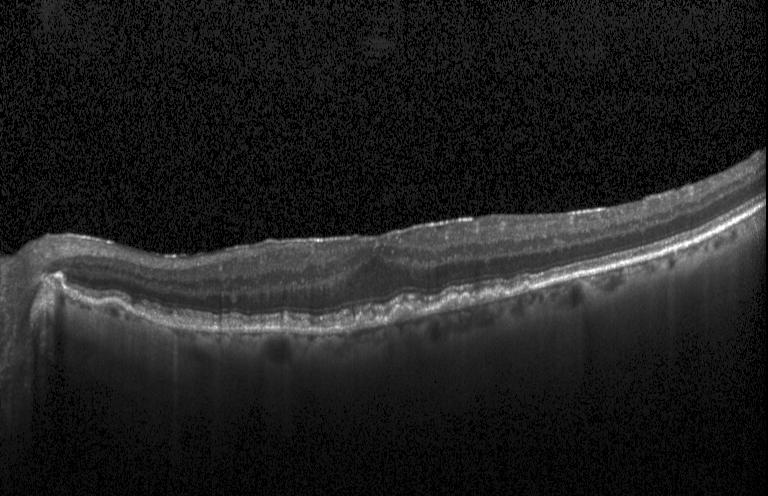
Optical coherence tomography B-scan · through the macula · Heidelberg Spectralis OCT system · spectral-domain OCT.
Diagnosis: a choroidal neovascular membrane.